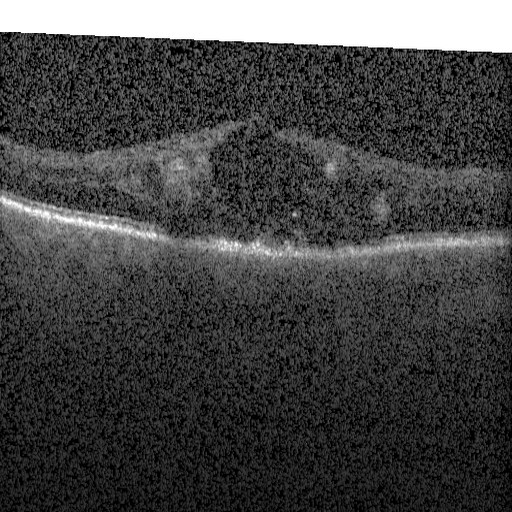 Macular OCT demonstrating diabetic macular edema (DME).